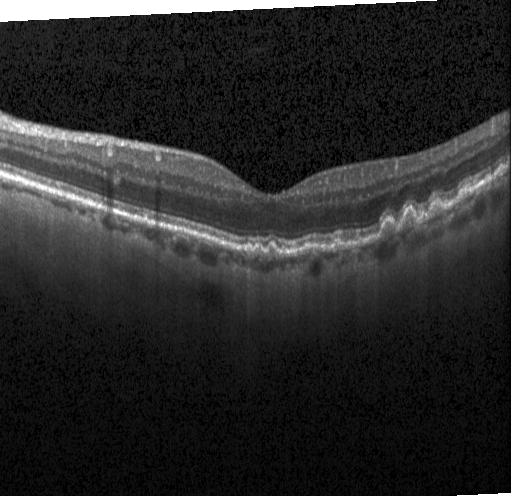
Through the macula. Heidelberg Spectralis. Spectral-domain optical coherence tomography. Retinal OCT B-scan — Dx: sub-RPE drusenoid deposits.